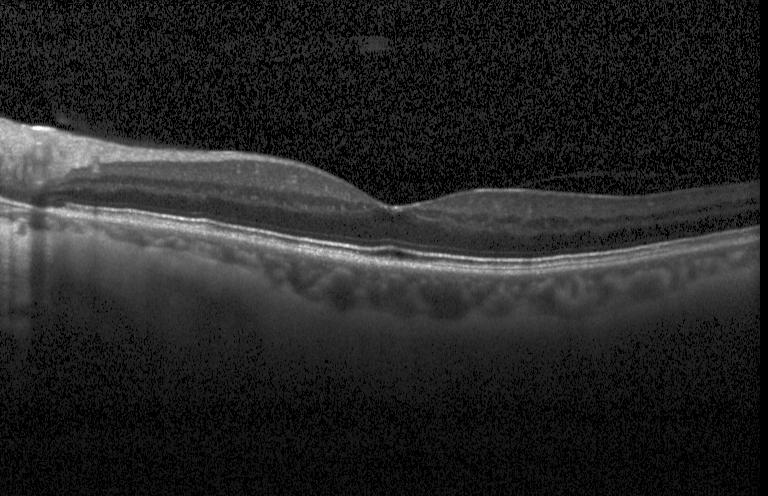
Fovea-centered; acquired on a Heidelberg Spectralis; OCT B-scan.
OCT finding: no choroidal neovascularization, diabetic macular edema, or drusen.